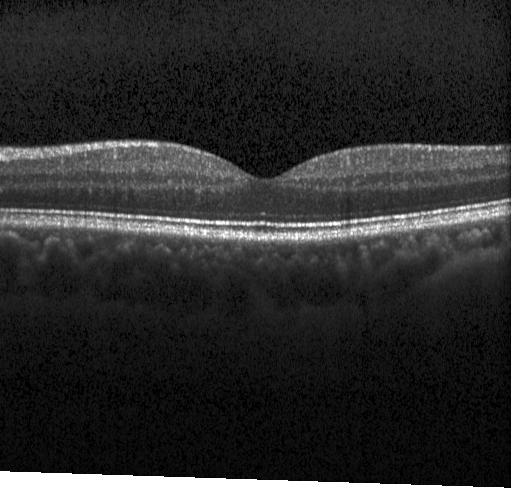
Instrument: Heidelberg Spectralis · SD-OCT · horizontal scan through the fovea · optical coherence tomography scan. OCT finding: no evidence of choroidal neovascularization, diabetic macular edema, or drusen.